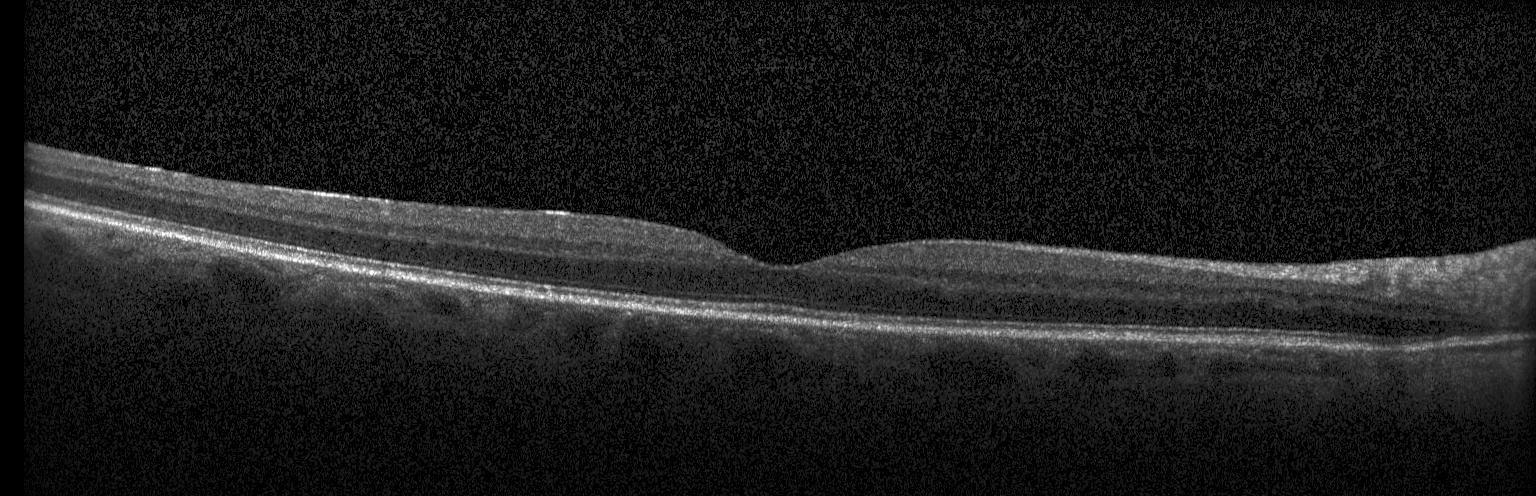
OCT line scan. Heidelberg Spectralis
Finding: neither CNV, DME, nor drusen.